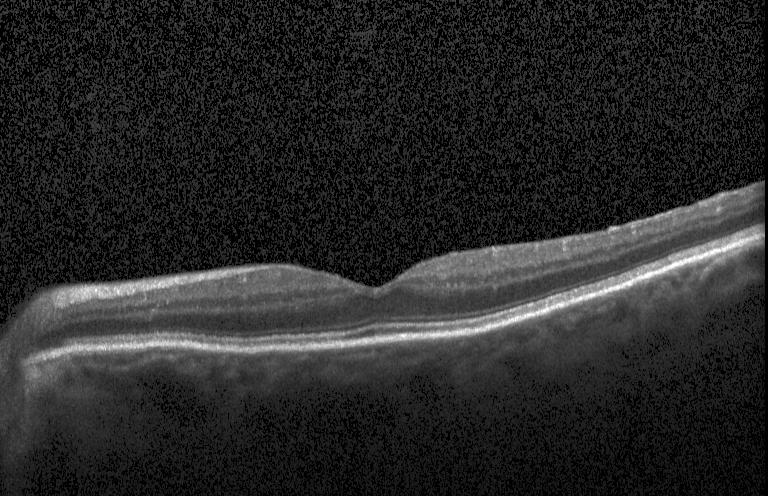 Retinal OCT B-scan. Horizontal scan through the fovea. Spectral-domain optical coherence tomography. Heidelberg Spectralis OCT system
Impression: neither choroidal neovascularization, diabetic macular edema, nor drusen.